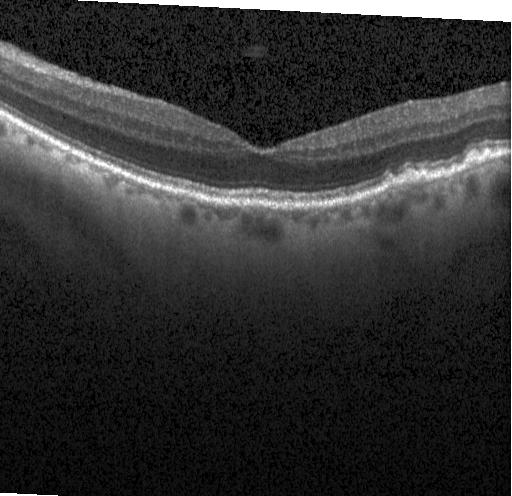

Heidelberg Spectralis · macular scan · SD-OCT · optical coherence tomography B-scan — This B-scan demonstrates drusen.